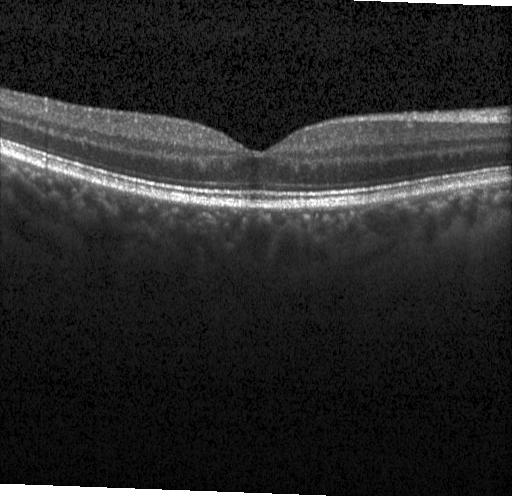 Spectral-domain OCT · through the macula · retinal OCT B-scan · Heidelberg Spectralis OCT system — Impression: no choroidal neovascularization, no diabetic macular edema, and no drusen.